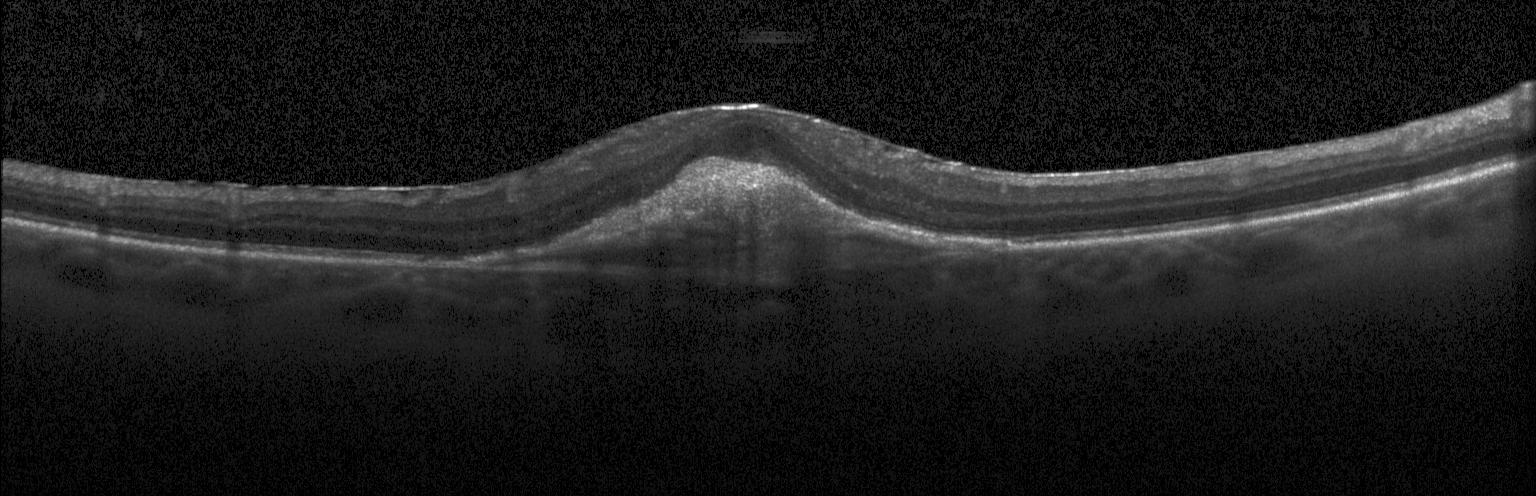 Horizontal scan through the fovea · Heidelberg Spectralis OCT system · optical coherence tomography scan.
Impression: a choroidal neovascular membrane.